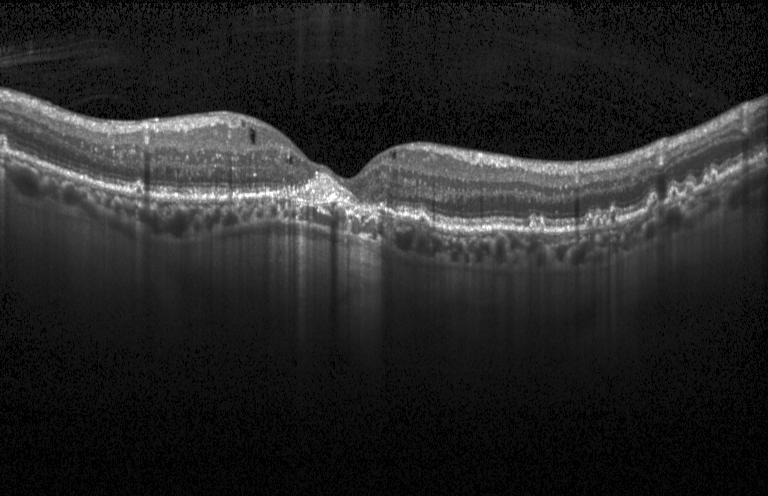
A choroidal neovascular membrane.